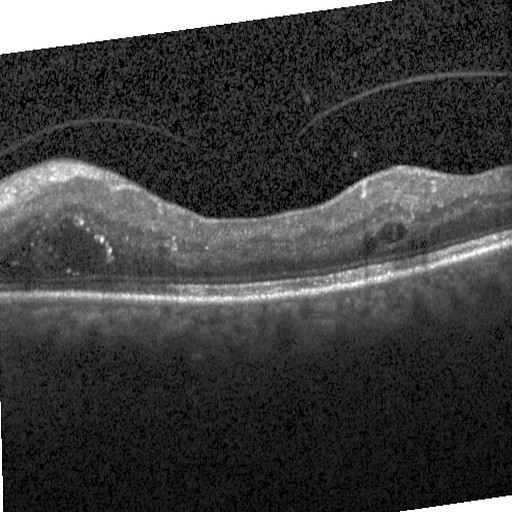
OCT B-scan showing DME.